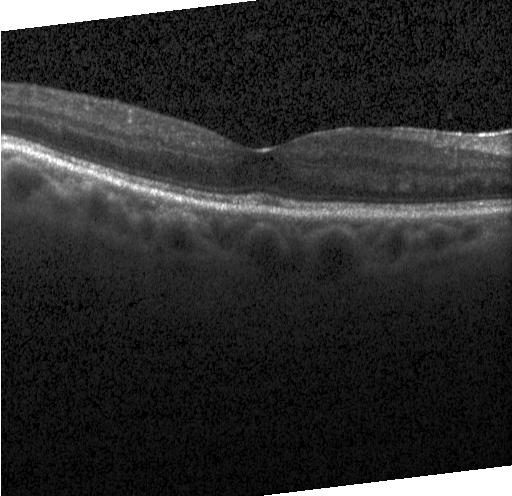 OCT scan showing no evidence of choroidal neovascularization, diabetic macular edema, or drusen.